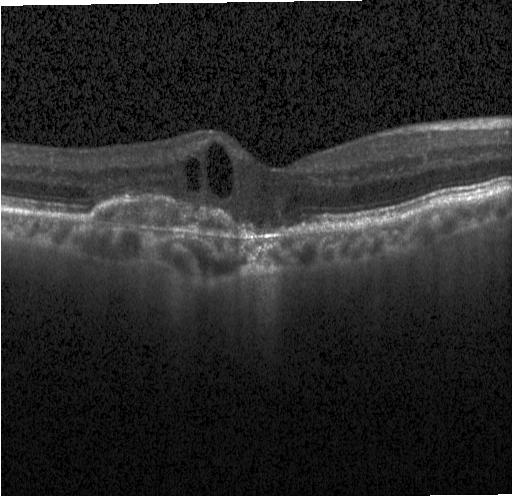

OCT B-scan, acquired on a Heidelberg Spectralis, macular scan, spectral-domain OCT.
OCT finding: a choroidal neovascular membrane.